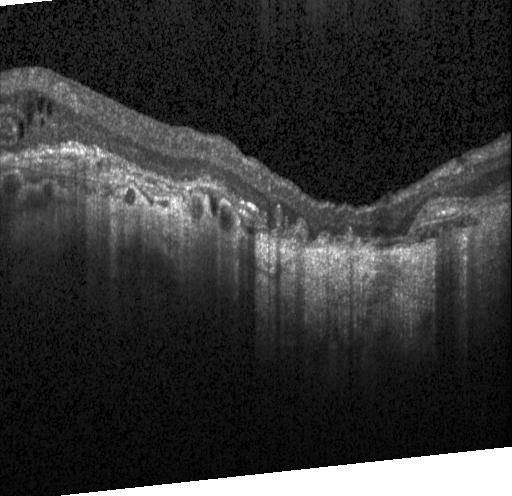

Optical coherence tomography scan — This B-scan demonstrates a choroidal neovascular membrane.